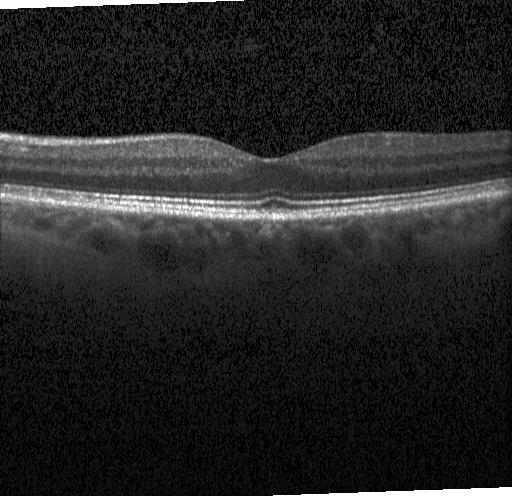 Retinal OCT B-scan.
Finding: no choroidal neovascularization, no diabetic macular edema, and no drusen.